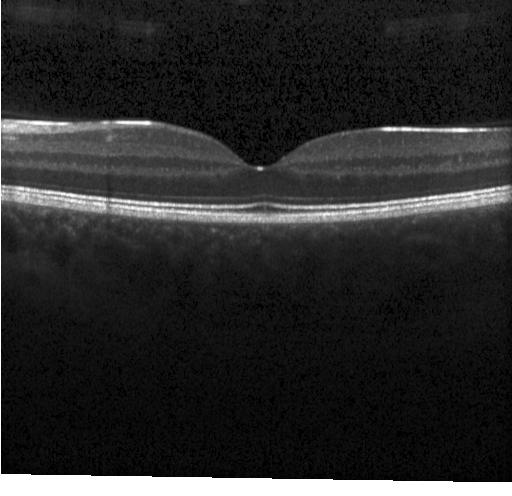 OCT line scan · SD-OCT
This B-scan demonstrates neither CNV, DME, nor drusen.